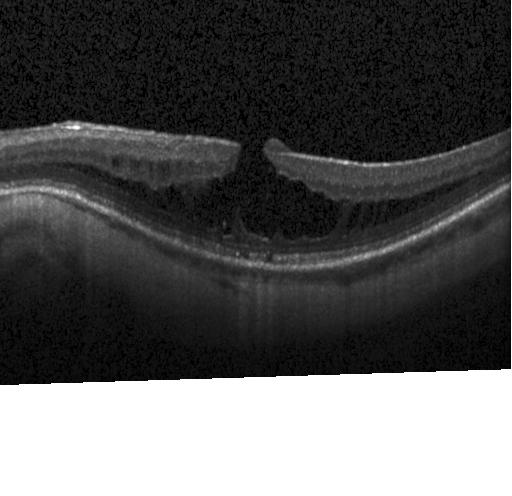 This B-scan demonstrates DME.